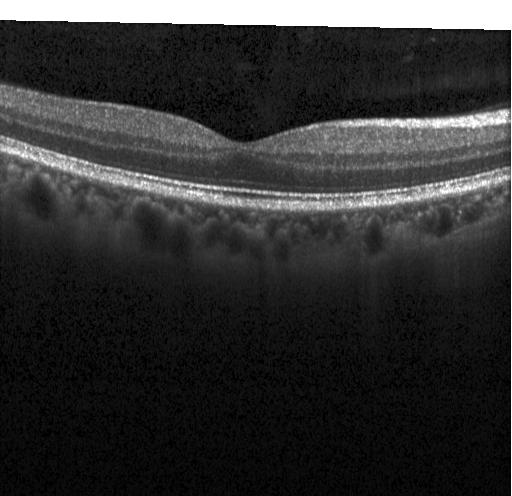 Retinal OCT cross-section
Finding: no CNV, DME, or drusen.